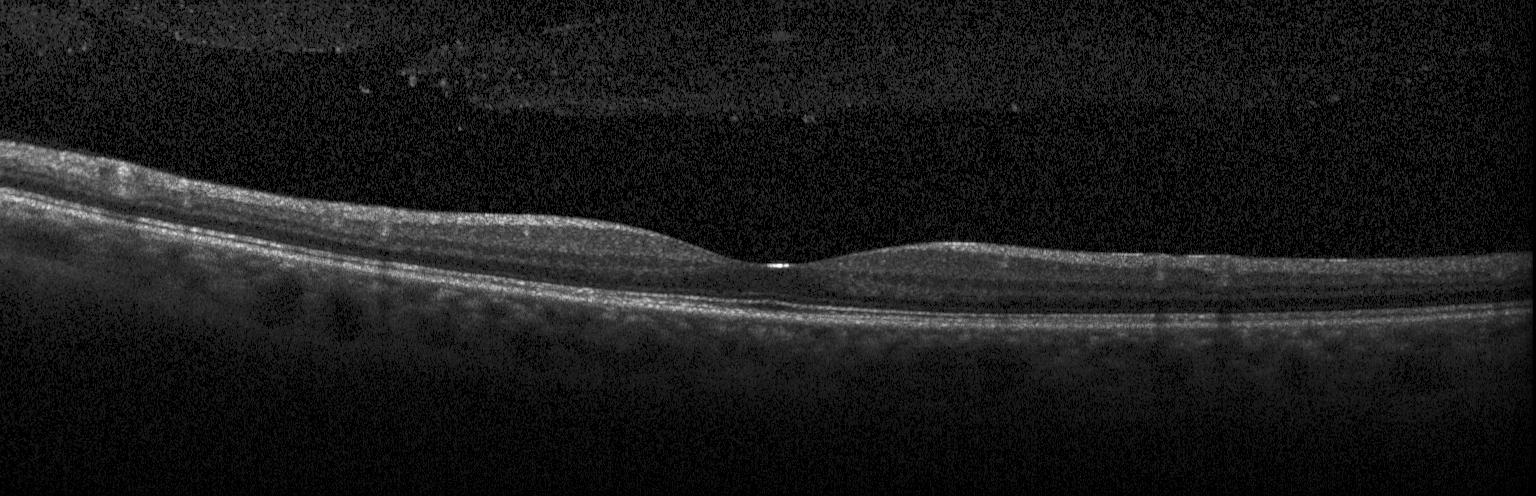

OCT line scan.
Impression: no evidence of choroidal neovascularization, diabetic macular edema, or drusen.